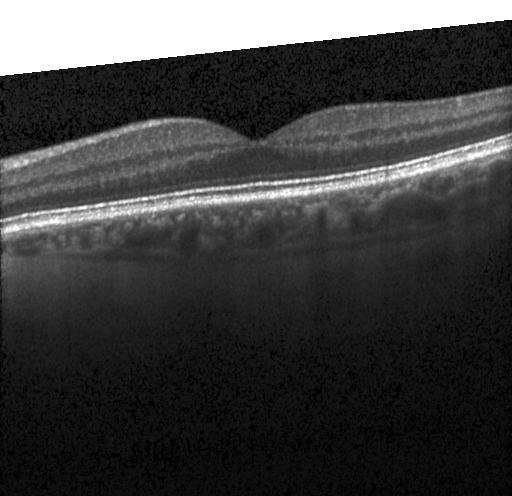

Dx: no CNV, DME, or drusen.